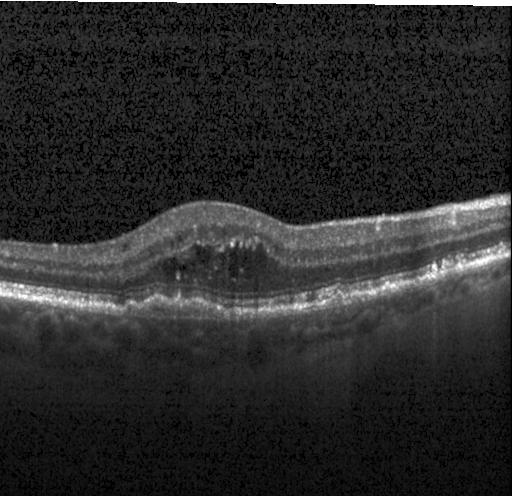 Retinal OCT cross-section.
Finding: choroidal neovascularization (CNV).